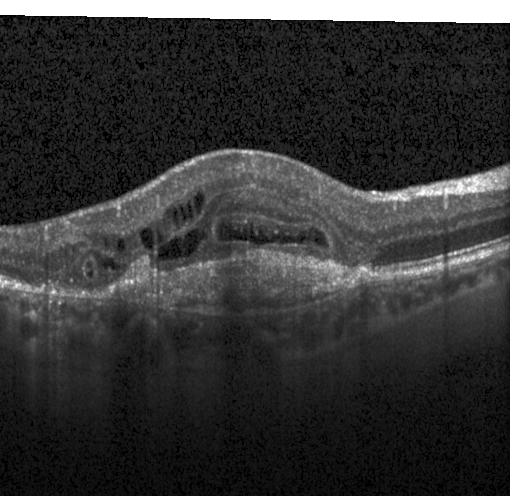 OCT line scan, macular scan, spectral-domain optical coherence tomography, instrument: Heidelberg Spectralis.
This B-scan demonstrates a choroidal neovascular membrane.